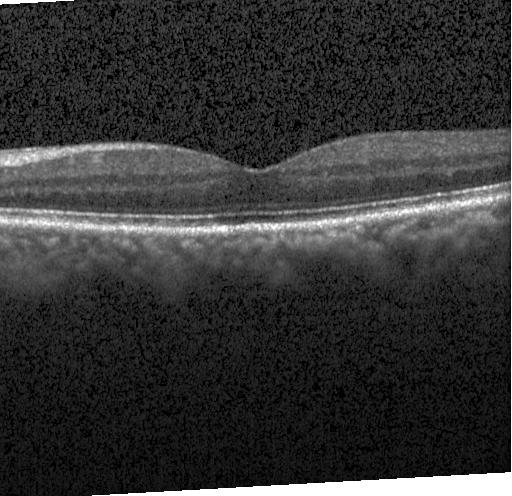 Impression: no evidence of CNV, DME, or drusen.